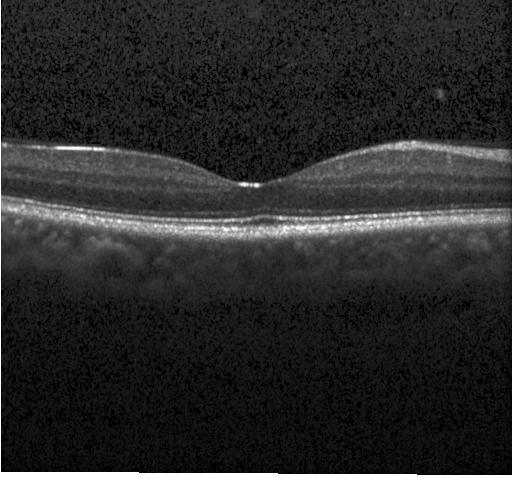 Fovea-centered, OCT B-scan — The scan shows neither choroidal neovascularization, diabetic macular edema, nor drusen.